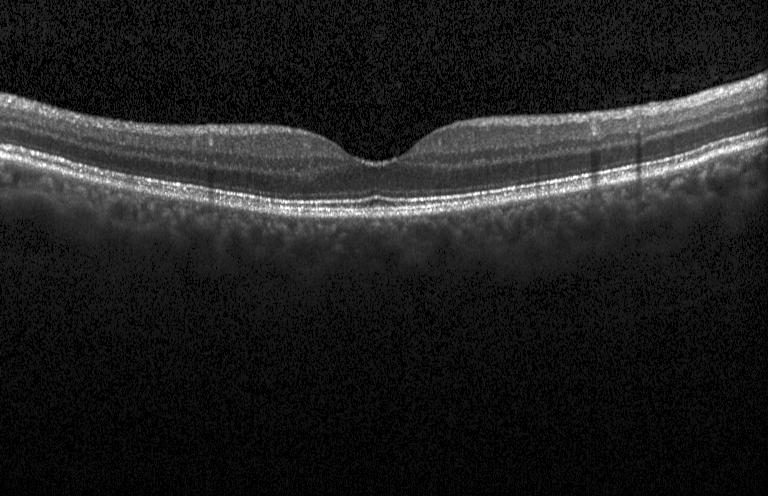 Finding: neither CNV, DME, nor drusen.